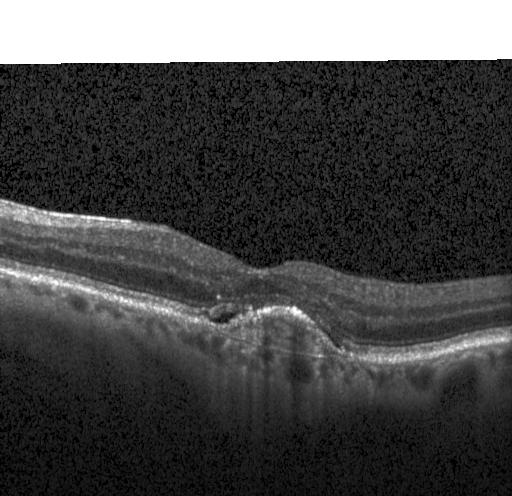 Through the macula; instrument: Heidelberg Spectralis; optical coherence tomography scan. Impression: a choroidal neovascular membrane.